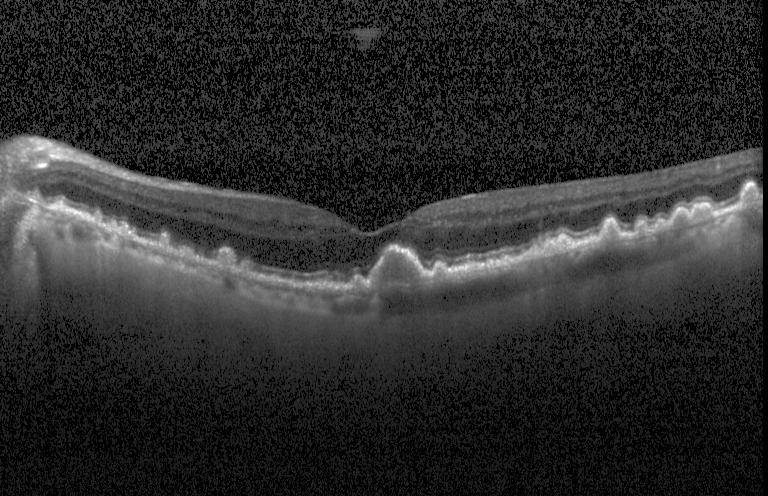
Sub-RPE drusenoid deposits.